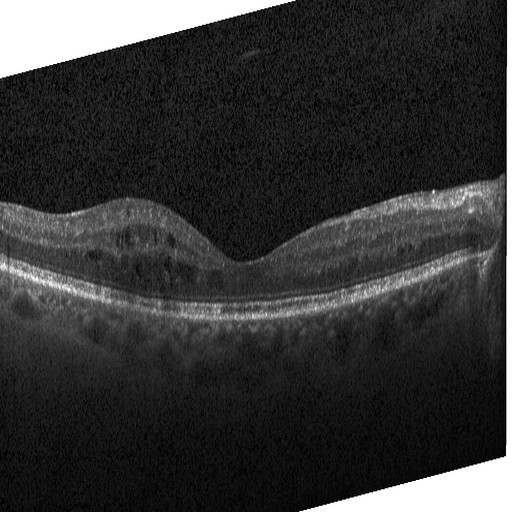 SD-OCT · optical coherence tomography scan. Diagnosis: diabetic macular edema (DME).